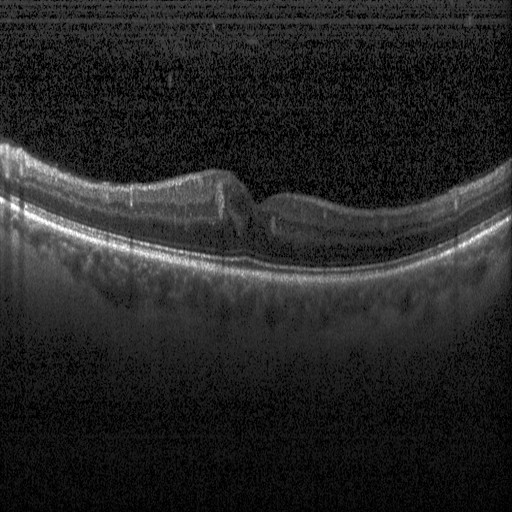
Retinal OCT cross-section; horizontal scan through the fovea; Heidelberg Spectralis OCT system.
Diagnosis: diabetic macular edema (DME).